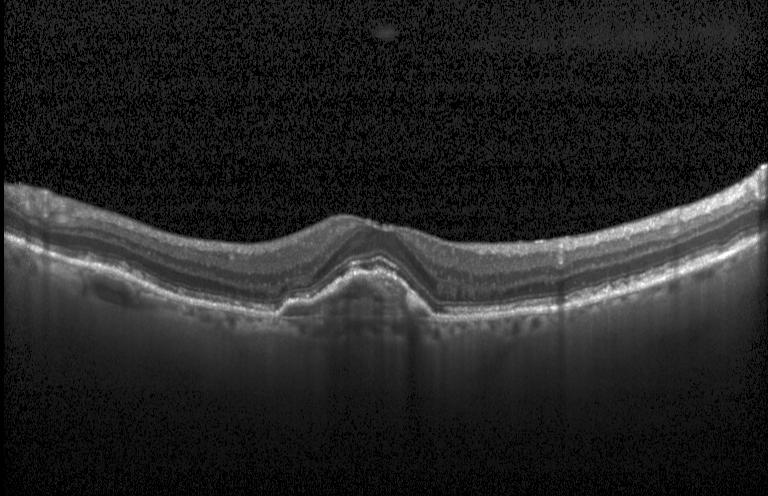
OCT line scan; spectral-domain OCT
This B-scan demonstrates choroidal neovascularization (CNV).